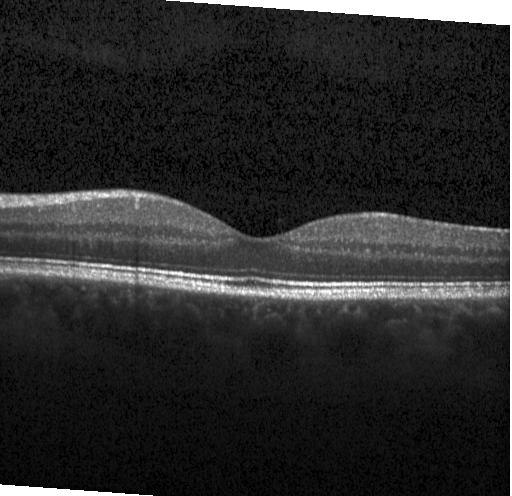 SD-OCT. Retinal OCT cross-section — Impression: no choroidal neovascularization, no diabetic macular edema, and no drusen.